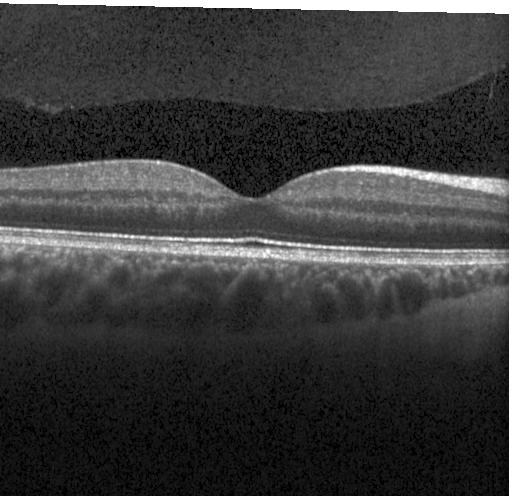
No evidence of CNV, DME, or drusen.